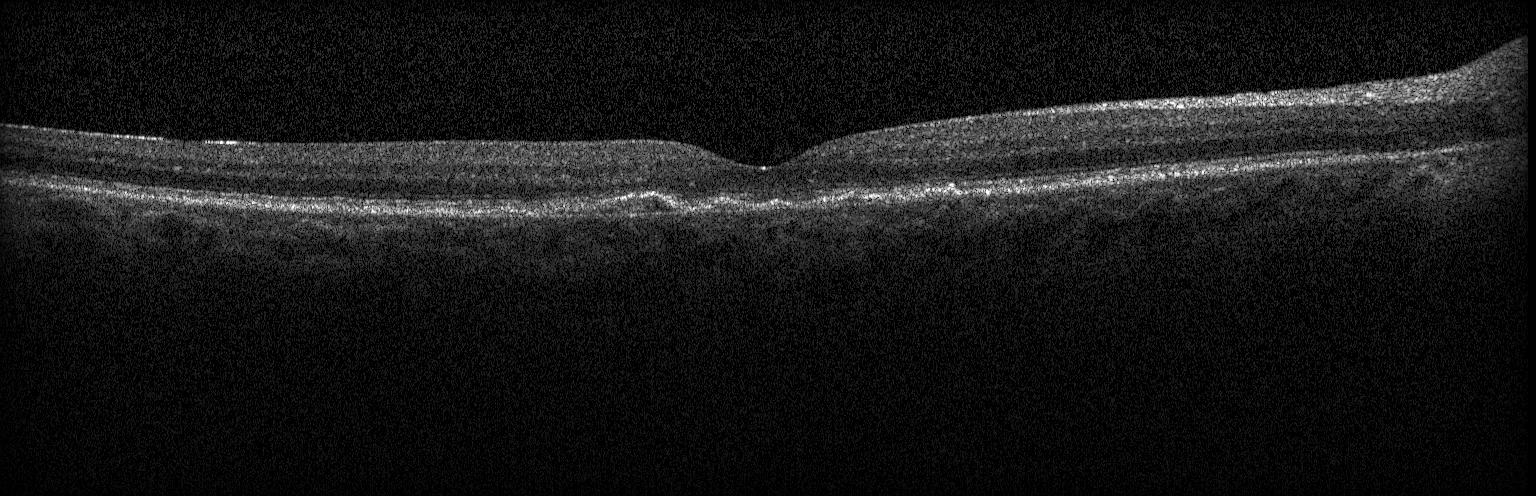
CNV.